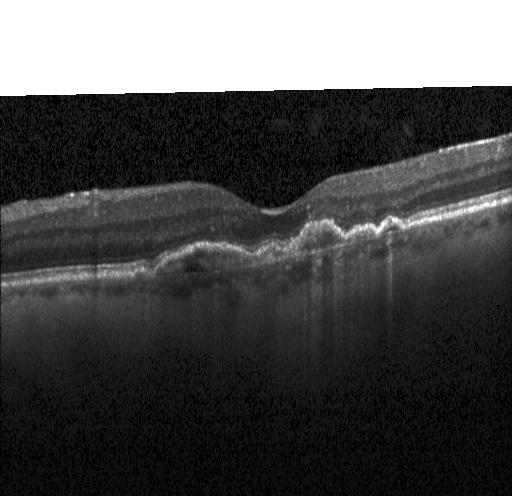
Diagnosis: a choroidal neovascular membrane.